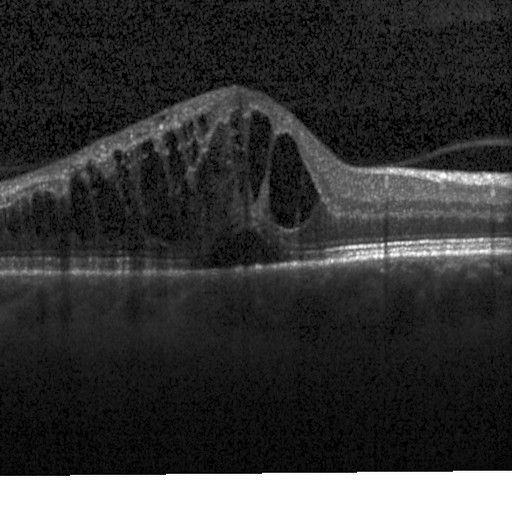 Optical coherence tomography B-scan. Spectral-domain optical coherence tomography. Acquired on a Heidelberg Spectralis.
Diabetic macular edema (DME).